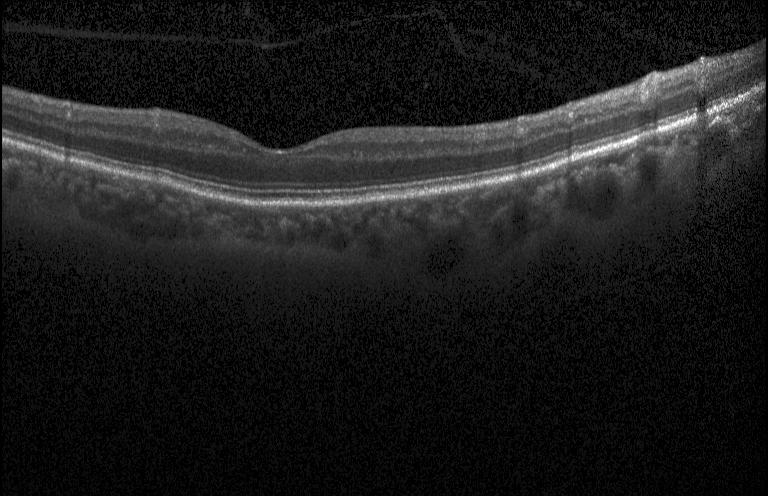 Spectral-domain OCT. Instrument: Heidelberg Spectralis. OCT line scan. Macular OCT: no evidence of choroidal neovascularization, diabetic macular edema, or drusen.